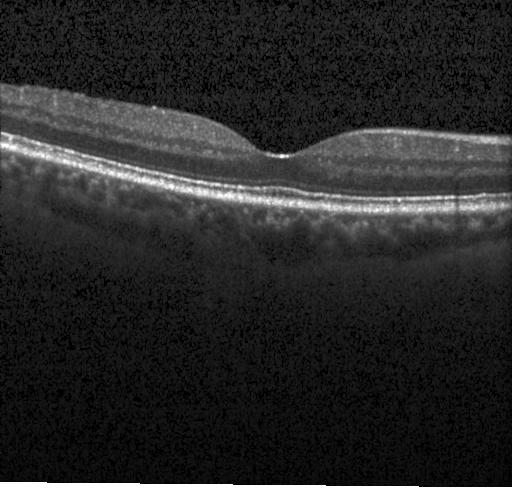

Fovea-centered. Optical coherence tomography scan. Acquired on a Heidelberg Spectralis. Diagnosis: no choroidal neovascularization, no diabetic macular edema, and no drusen.